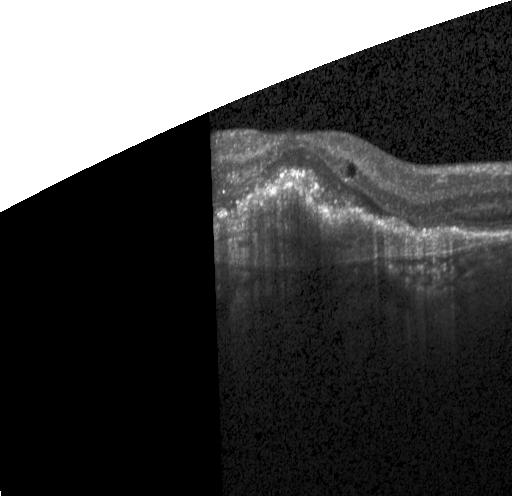
A choroidal neovascular membrane.